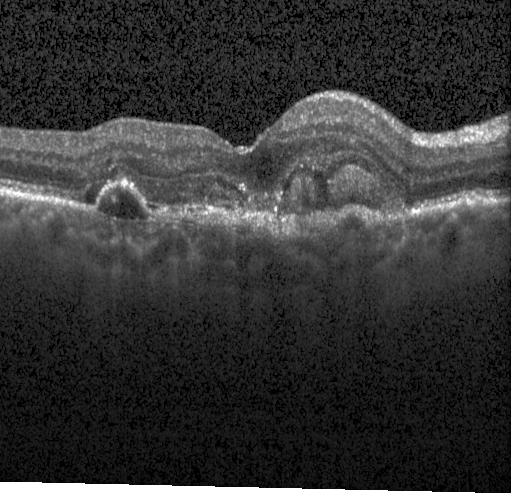

Dx: choroidal neovascularization.